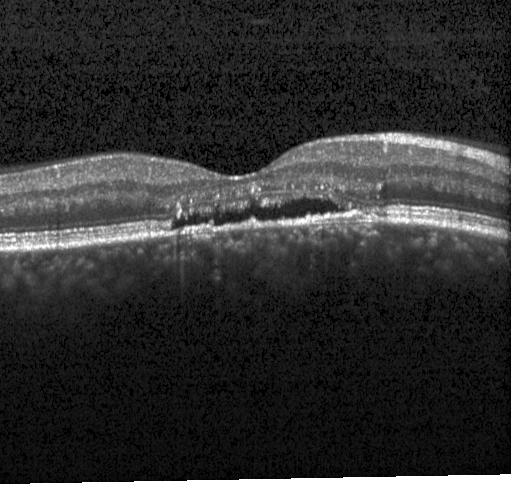

SD-OCT · OCT line scan · centered on the fovea · Heidelberg Spectralis — This B-scan demonstrates choroidal neovascularization.